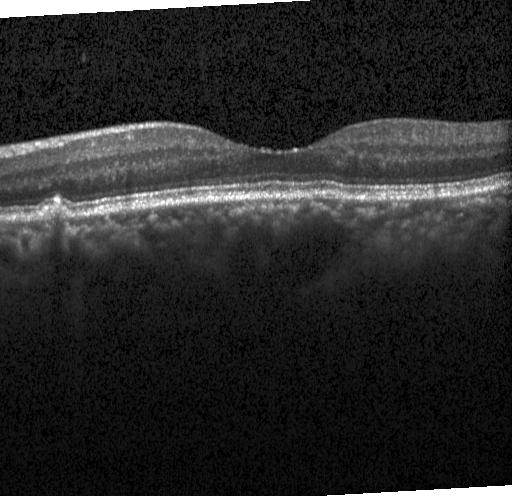

Spectral-domain OCT, optical coherence tomography scan, Heidelberg Spectralis, macular scan.
Dx: multiple drusen.